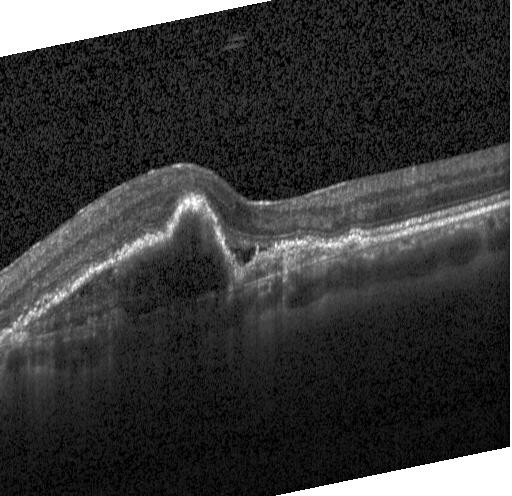 Retinal OCT cross-section, spectral-domain optical coherence tomography
The scan shows choroidal neovascularization.